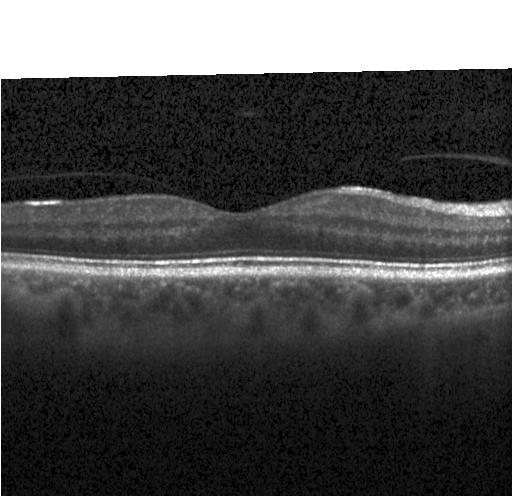 OCT line scan, spectral-domain OCT, fovea-centered, Heidelberg Spectralis OCT system. Assessment: no CNV, DME, or drusen.